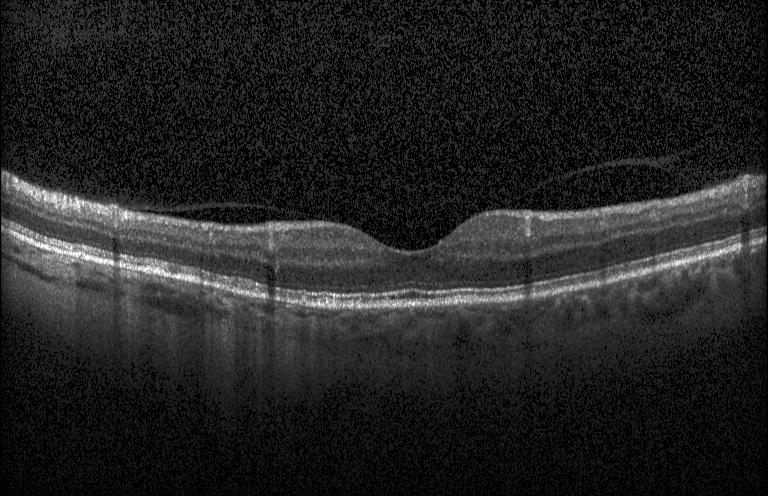 Optical coherence tomography B-scan, SD-OCT
Diagnosis: no evidence of choroidal neovascularization, diabetic macular edema, or drusen.